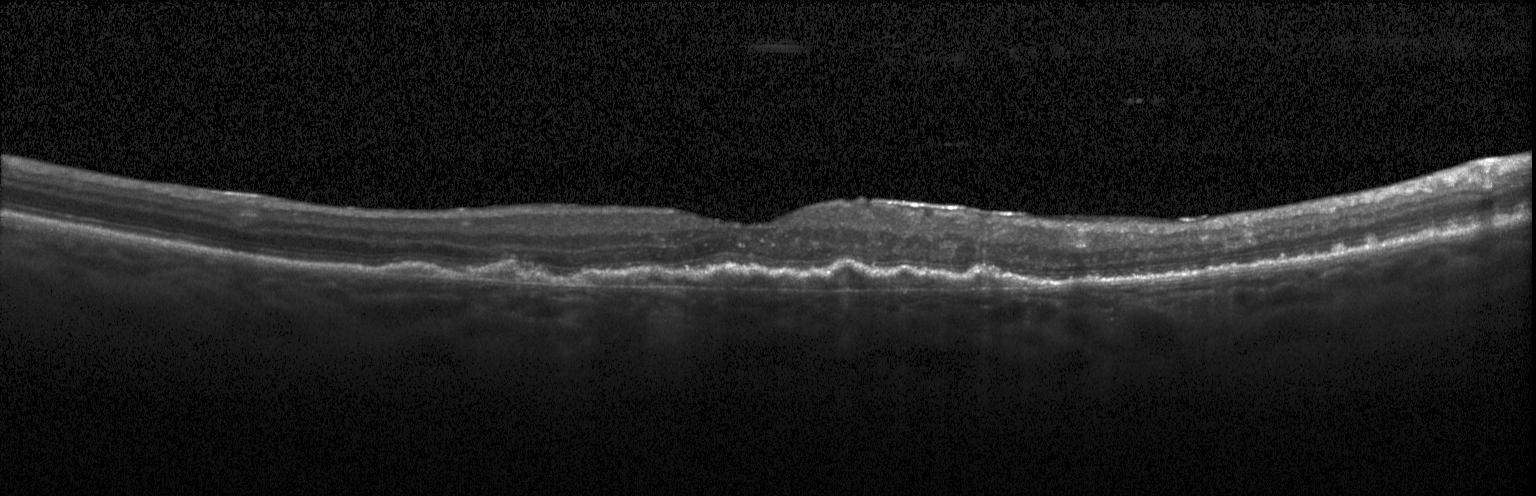 Spectral-domain OCT B-scan: a choroidal neovascular membrane.